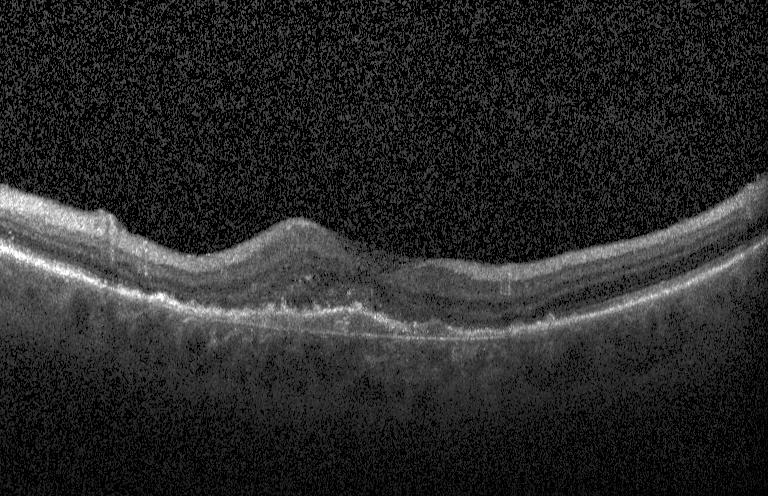

Impression: a choroidal neovascular membrane.